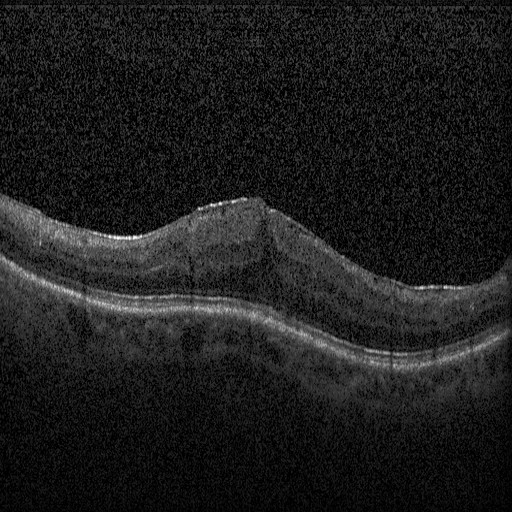
Dx: diabetic macular edema (DME).